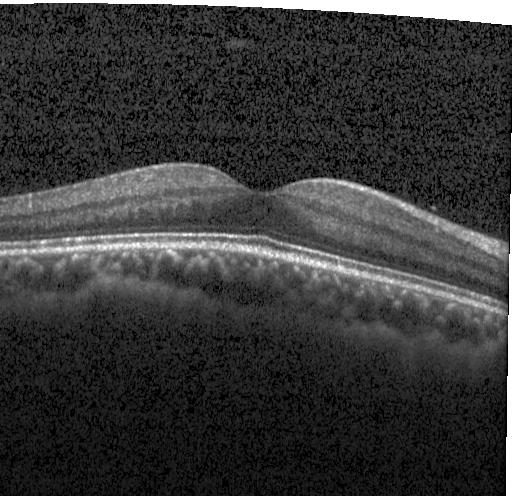 OCT line scan. Impression: no evidence of choroidal neovascularization, diabetic macular edema, or drusen.